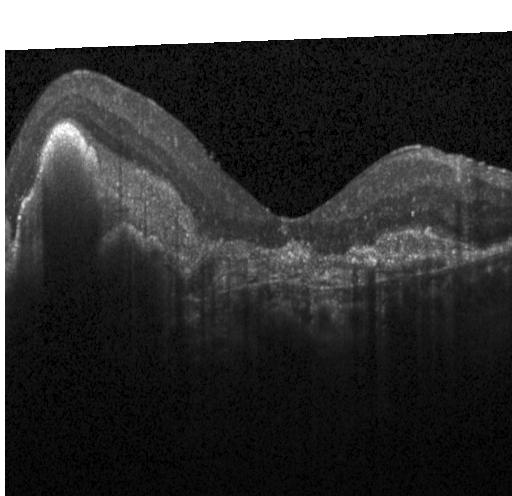

Impression: choroidal neovascularization.